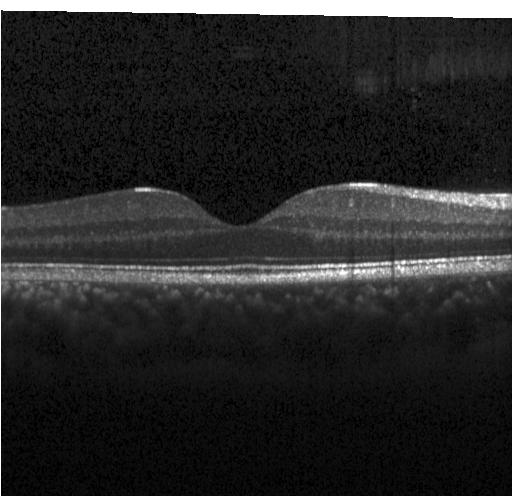
OCT line scan.
Assessment: no evidence of choroidal neovascularization, diabetic macular edema, or drusen.